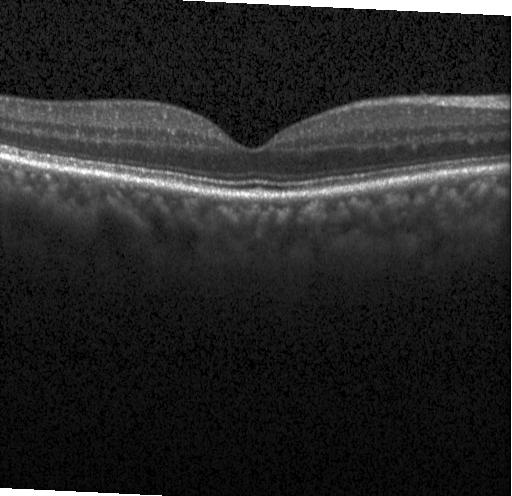 Through the macula; OCT B-scan; acquired on a Heidelberg Spectralis. Assessment: no choroidal neovascularization, no diabetic macular edema, and no drusen.